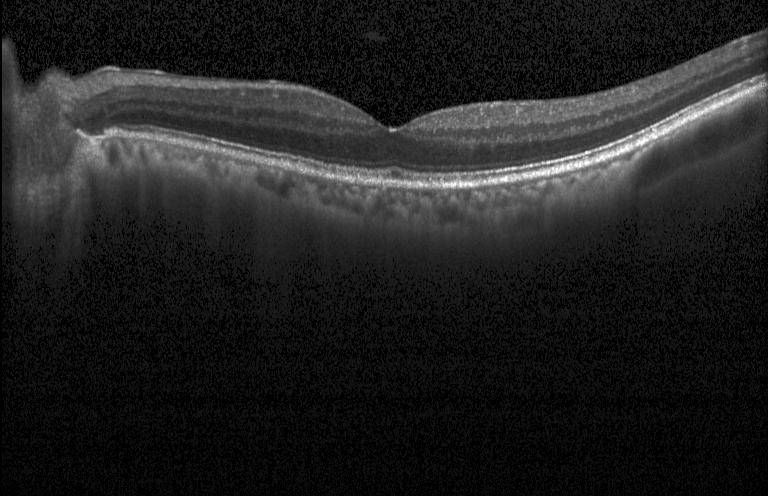

Acquired on a Heidelberg Spectralis, optical coherence tomography B-scan, fovea-centered. Diagnosis: neither choroidal neovascularization, diabetic macular edema, nor drusen.